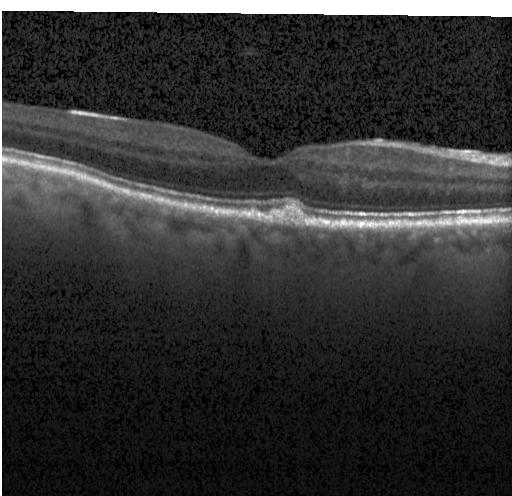 Acquired on a Heidelberg Spectralis; retinal OCT cross-section.
Assessment: sub-RPE drusenoid deposits.